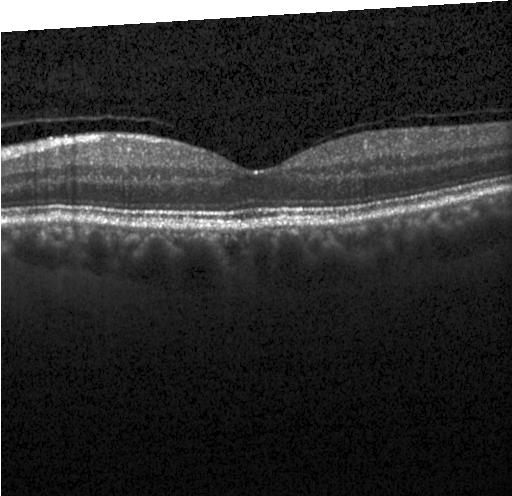
Impression: no evidence of choroidal neovascularization, diabetic macular edema, or drusen.